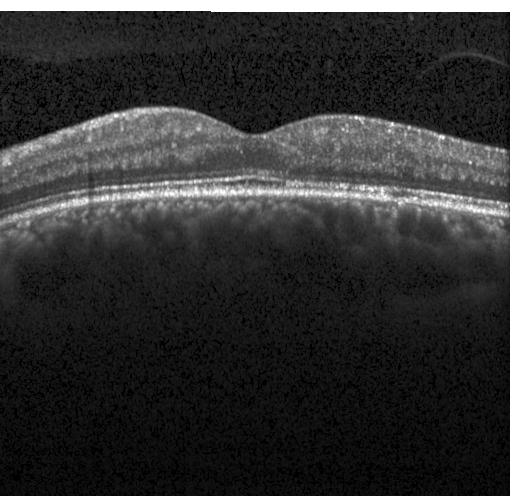

The scan shows no choroidal neovascularization, diabetic macular edema, or drusen.